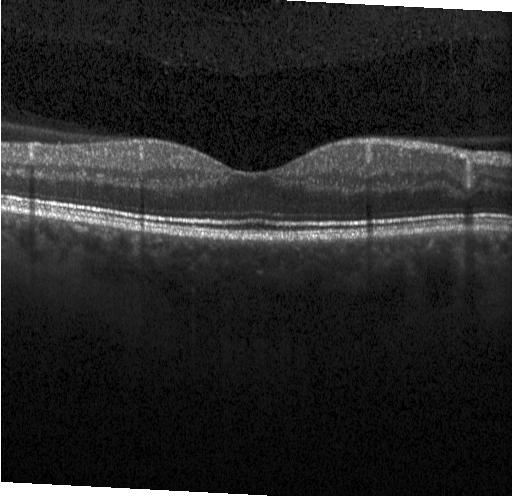

OCT finding: no choroidal neovascularization, diabetic macular edema, or drusen.